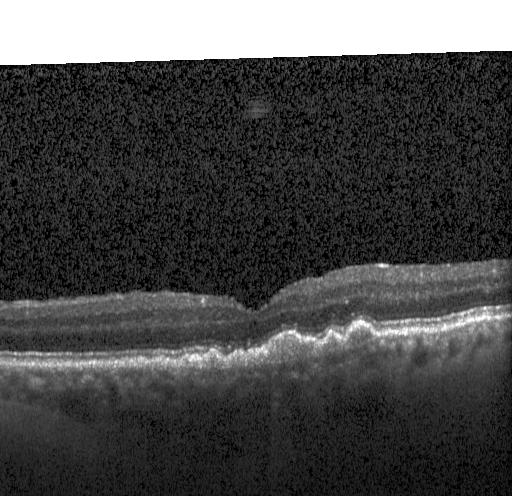

Heidelberg Spectralis, OCT line scan, horizontal scan through the fovea.
Dx: sub-RPE drusenoid deposits.